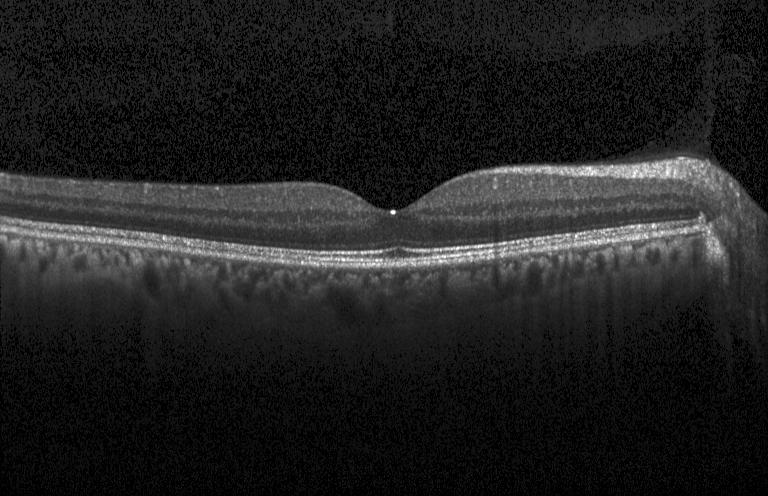

Finding: no choroidal neovascularization, diabetic macular edema, or drusen.